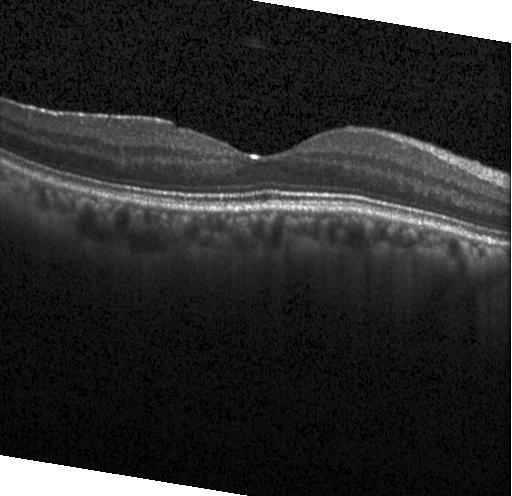 Horizontal scan through the fovea · OCT line scan · Heidelberg Spectralis OCT system.
OCT finding: no CNV, DME, or drusen.